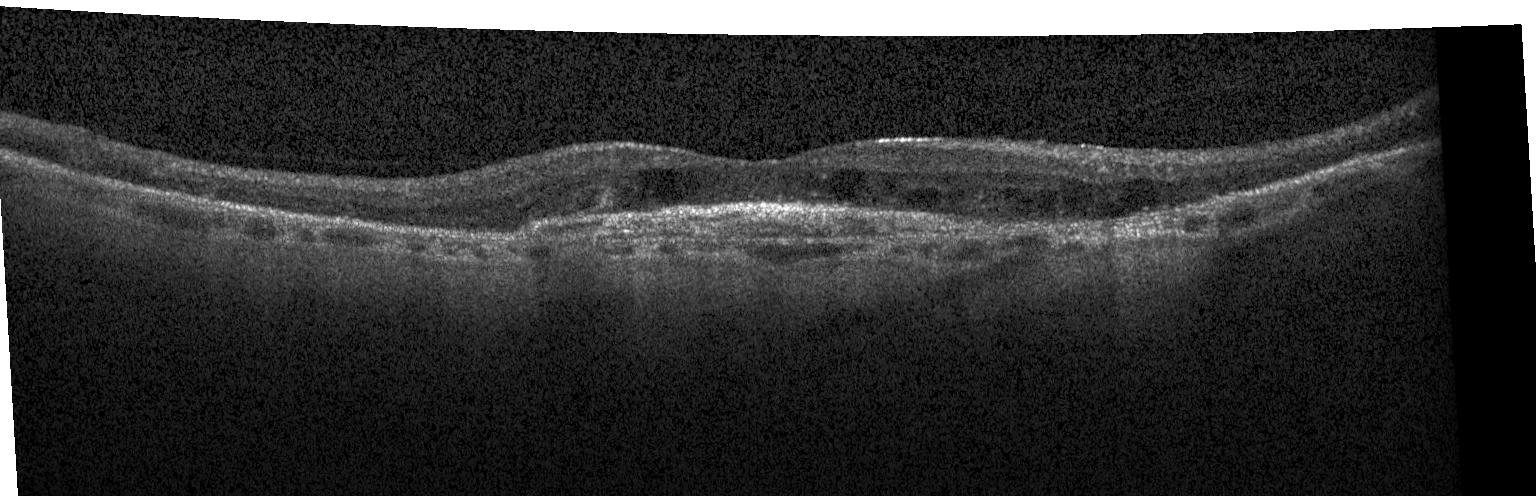

Horizontal scan through the fovea · Heidelberg Spectralis OCT system · OCT line scan
OCT finding: a choroidal neovascular membrane.